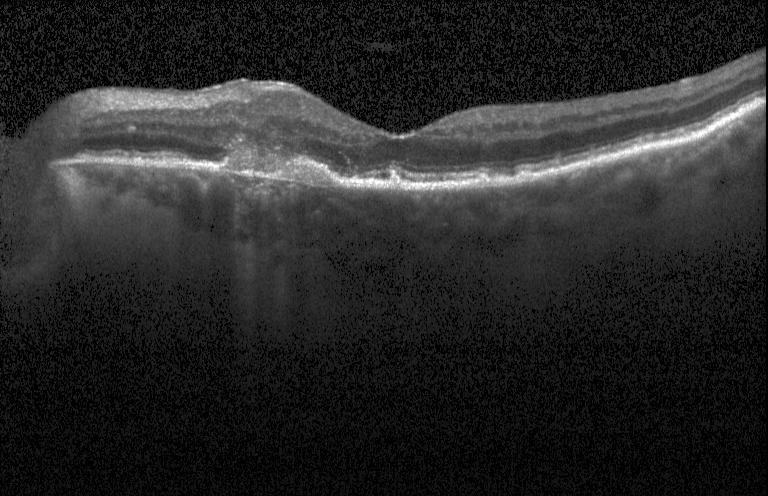 Diagnosis: a choroidal neovascular membrane.